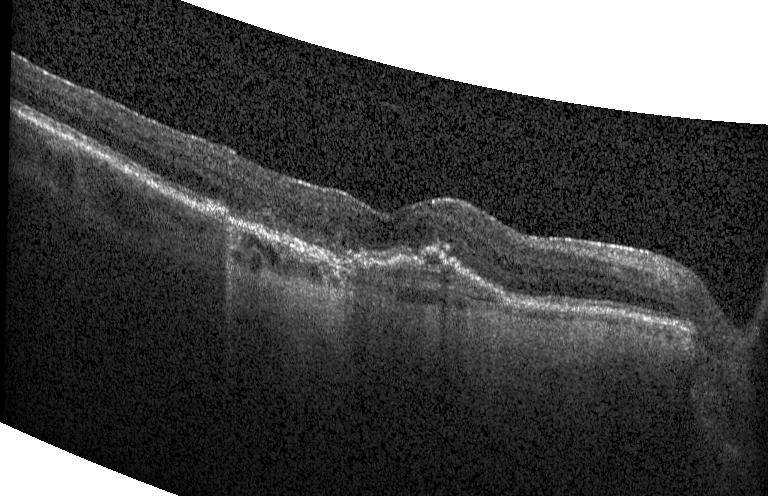

CNV.